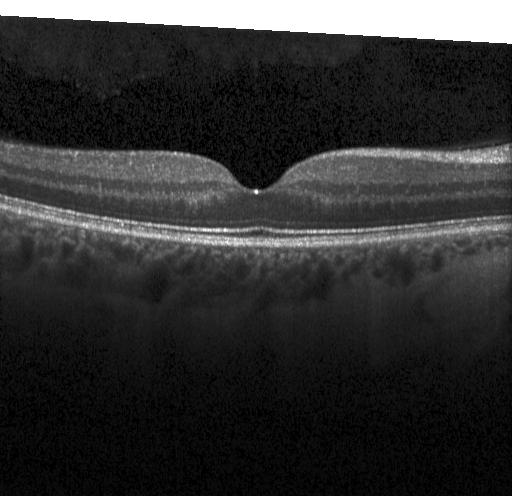

Instrument: Heidelberg Spectralis · spectral-domain OCT · optical coherence tomography scan · through the macula
Assessment: no evidence of choroidal neovascularization, diabetic macular edema, or drusen.